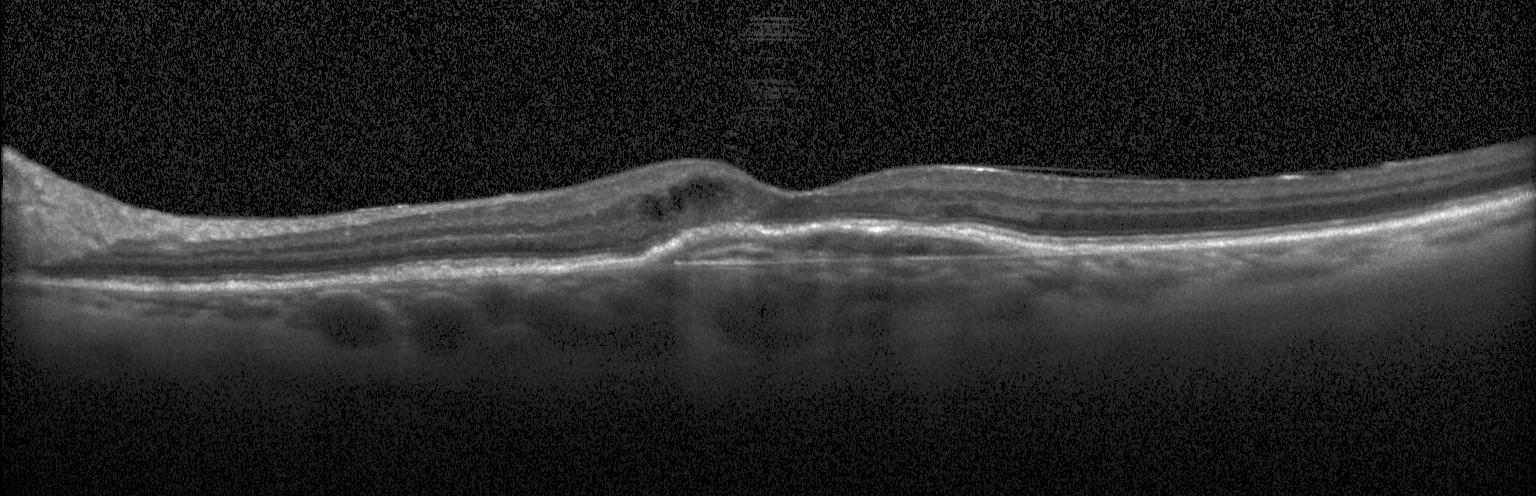
Spectral-domain OCT B-scan: choroidal neovascularization (CNV).